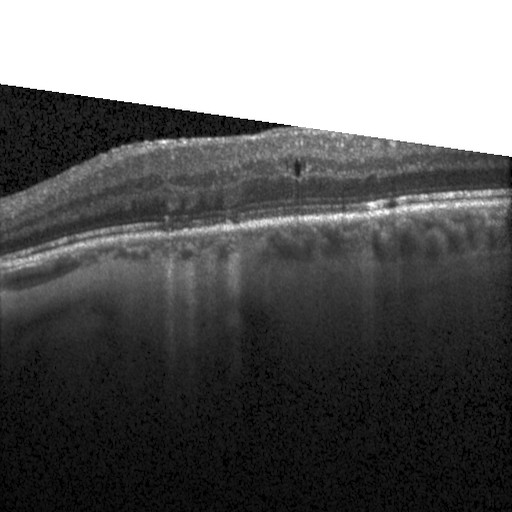 Optical coherence tomography scan; Heidelberg Spectralis OCT system; spectral-domain OCT; centered on the fovea. Impression: diabetic macular edema (DME).